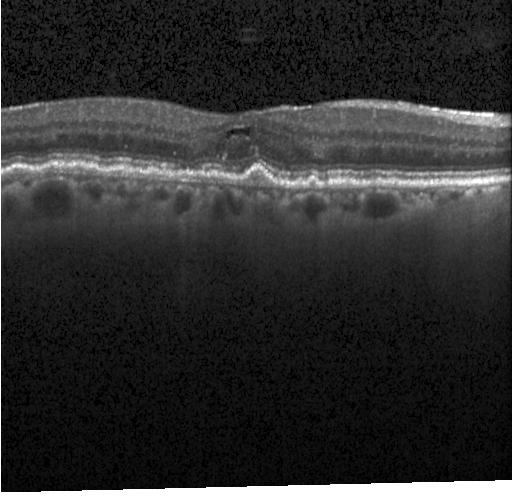

Retinal OCT B-scan, acquired on a Heidelberg Spectralis, fovea-centered, SD-OCT — OCT finding: choroidal neovascularization.